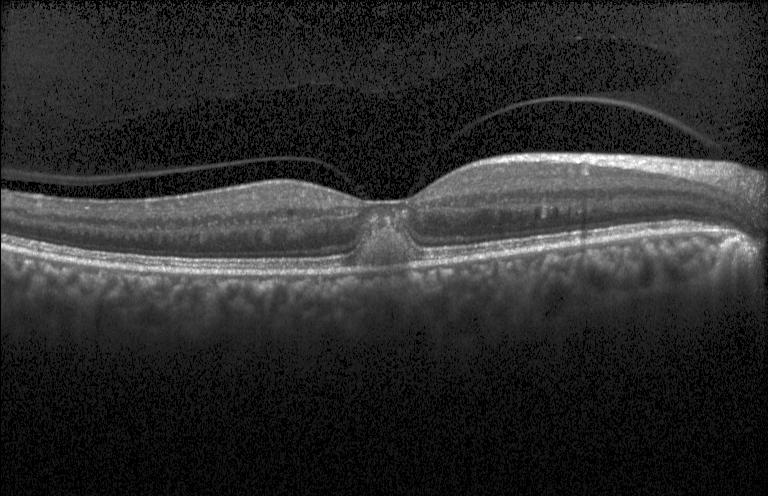 Acquired on a Heidelberg Spectralis, retinal OCT B-scan, SD-OCT, centered on the fovea — Assessment: CNV.